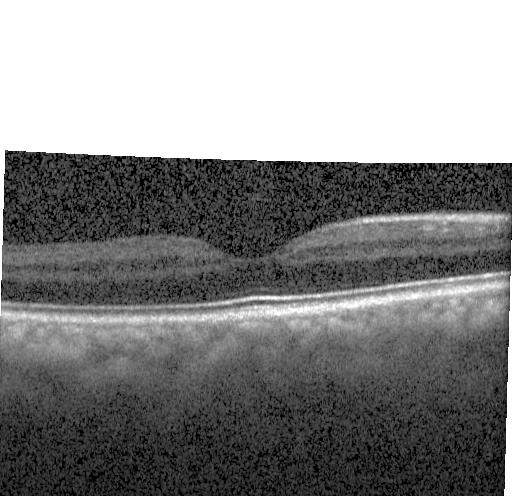 Horizontal scan through the fovea. Acquired on a Heidelberg Spectralis. Spectral-domain OCT. Optical coherence tomography scan.
Finding: neither CNV, DME, nor drusen.